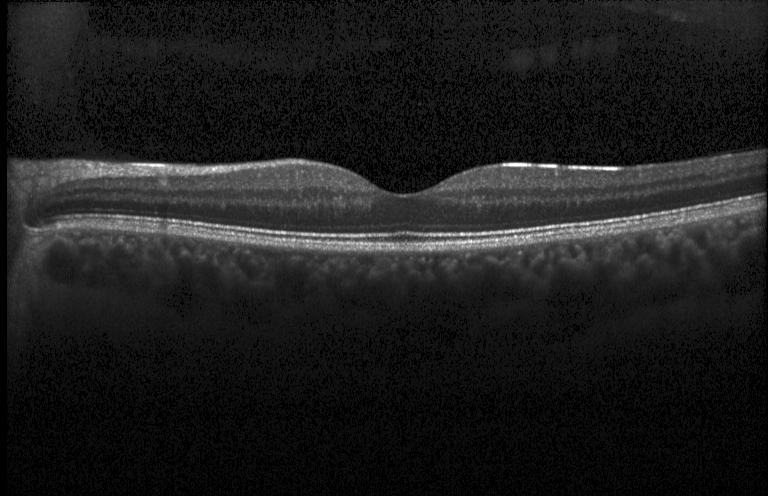 Instrument: Heidelberg Spectralis. Retinal OCT cross-section.
Diagnosis: no evidence of choroidal neovascularization, diabetic macular edema, or drusen.